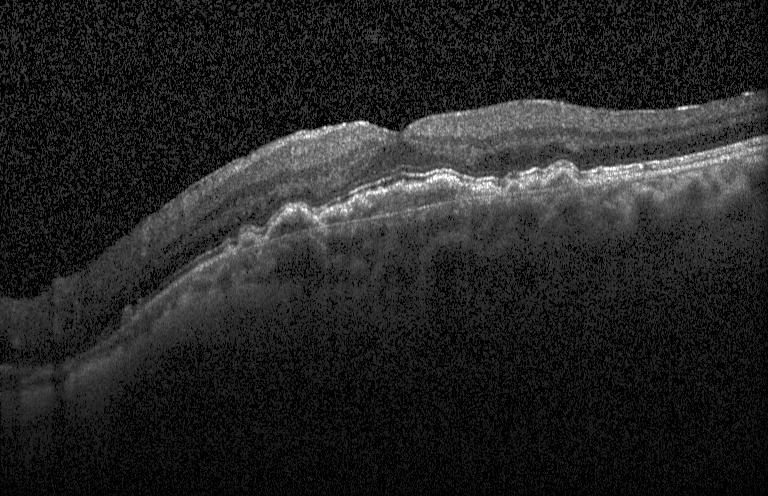 Optical coherence tomography B-scan. Dx: a choroidal neovascular membrane.